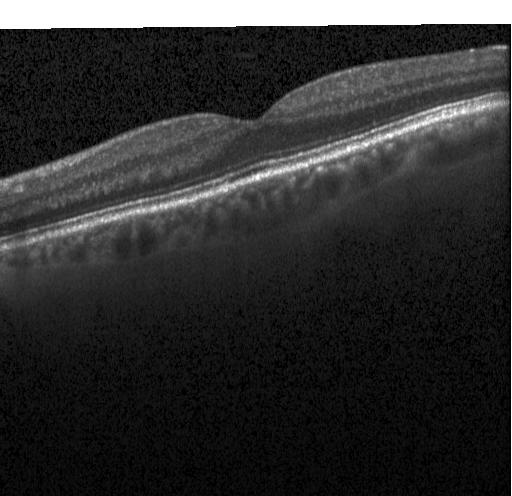
OCT B-scan; acquired on a Heidelberg Spectralis; macular scan; spectral-domain OCT. Assessment: no CNV, no DME, and no drusen.